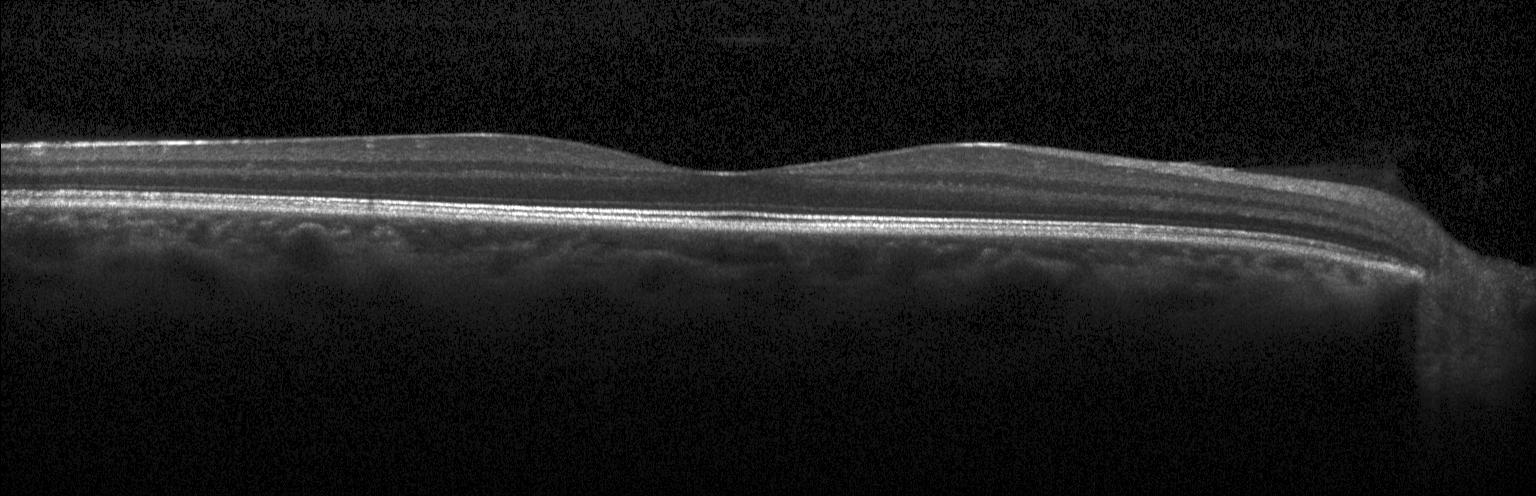 This B-scan demonstrates no evidence of choroidal neovascularization, diabetic macular edema, or drusen.